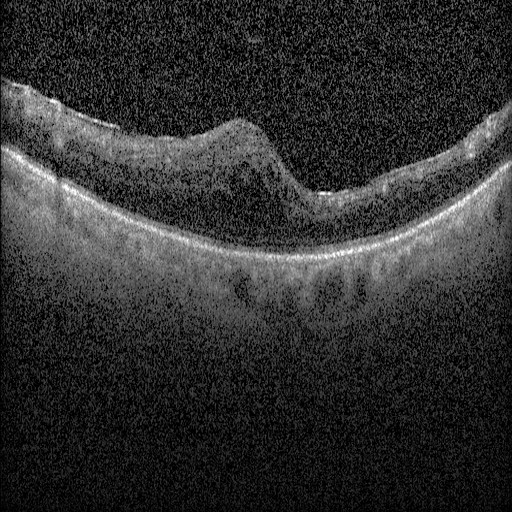 Macular OCT demonstrating diabetic macular edema.